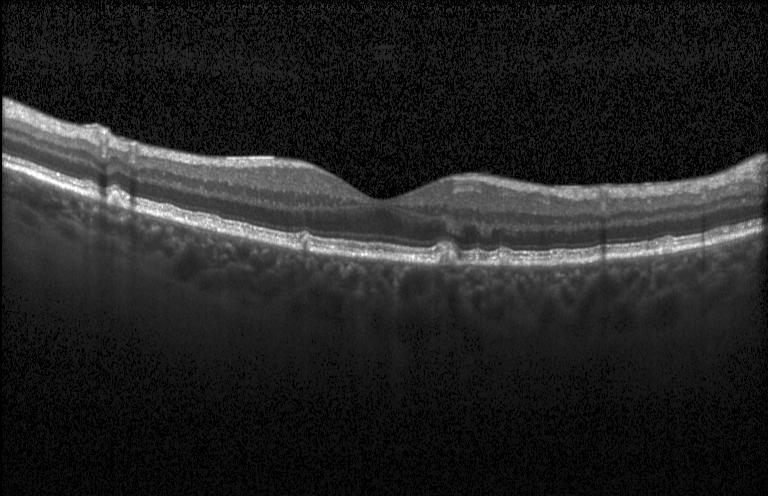
Finding: multiple drusen.